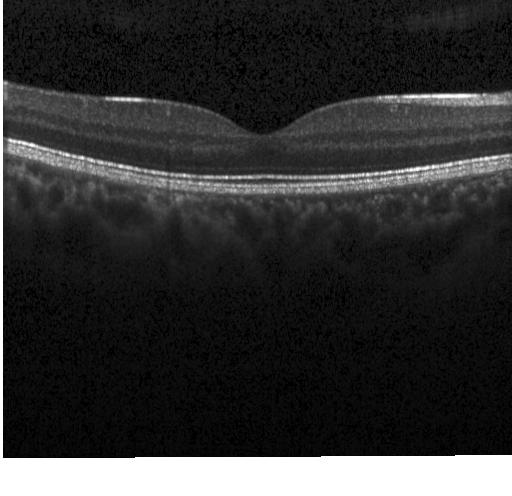 OCT scan showing no choroidal neovascularization, no diabetic macular edema, and no drusen.